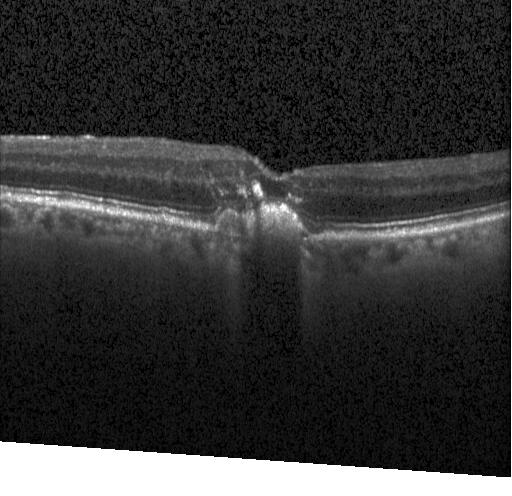 Optical coherence tomography B-scan. Impression: a choroidal neovascular membrane.